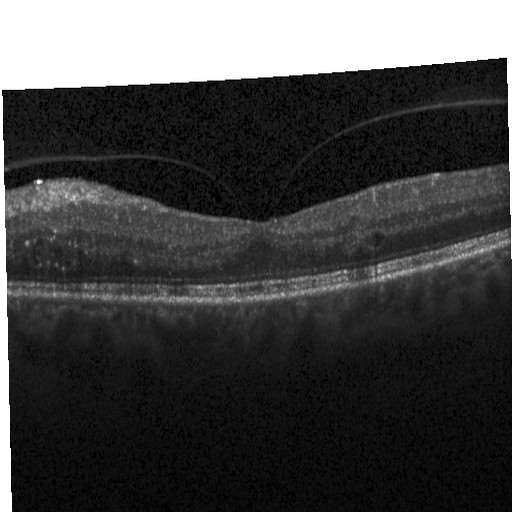
Instrument: Heidelberg Spectralis · SD-OCT · retinal OCT cross-section · centered on the fovea
Finding: diabetic macular edema.